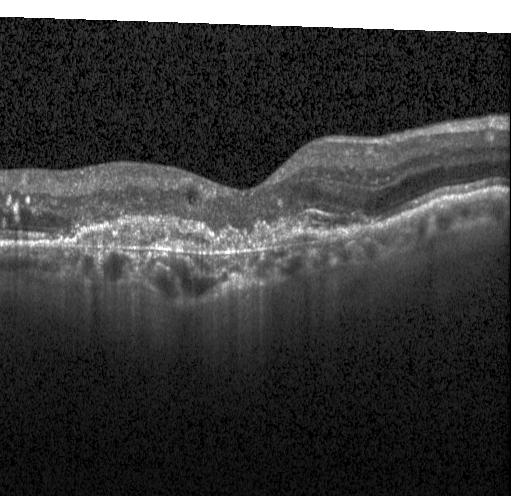

Heidelberg Spectralis OCT system · retinal OCT cross-section. Impression: choroidal neovascularization (CNV).